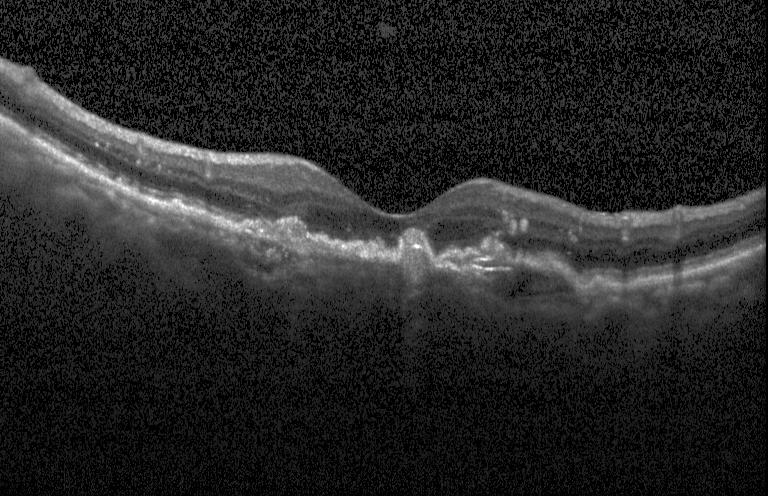

OCT line scan; spectral-domain optical coherence tomography. Diagnosis: choroidal neovascularization.